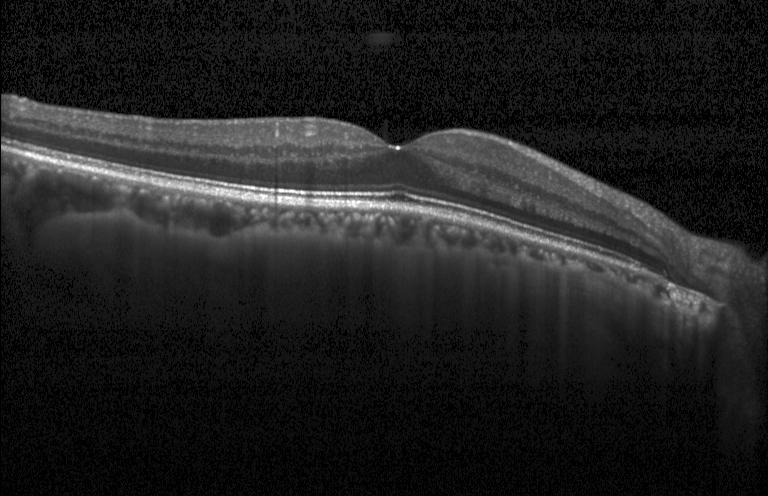

SD-OCT; Heidelberg Spectralis OCT system; OCT line scan; macular scan.
Finding: no evidence of choroidal neovascularization, diabetic macular edema, or drusen.